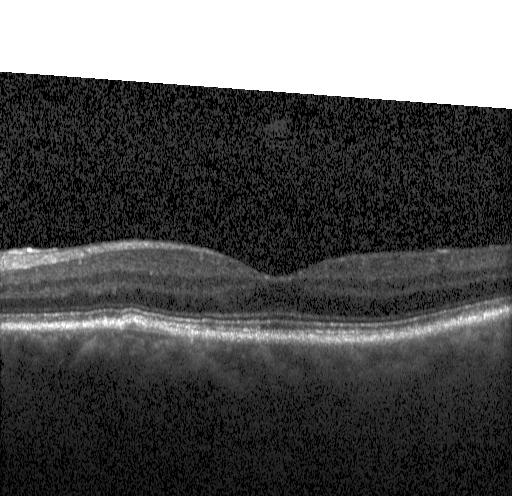 This B-scan demonstrates sub-RPE drusenoid deposits.